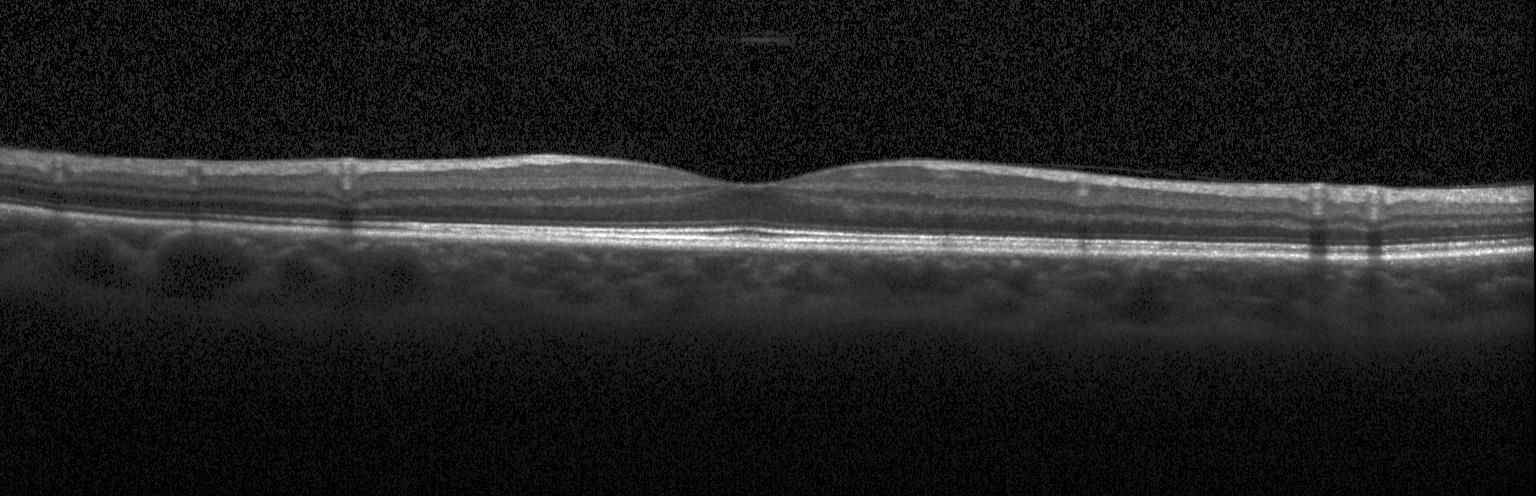
Retinal OCT B-scan · fovea-centered · SD-OCT · Heidelberg Spectralis OCT system. This B-scan demonstrates no evidence of choroidal neovascularization, diabetic macular edema, or drusen.